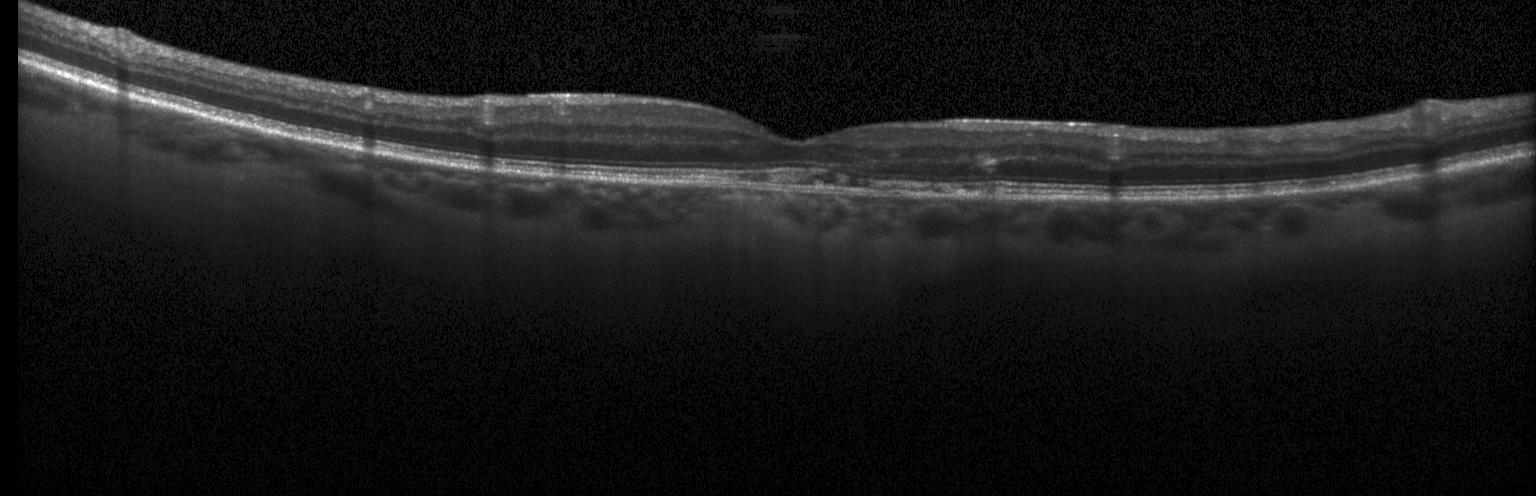
Diagnosis: a choroidal neovascular membrane.